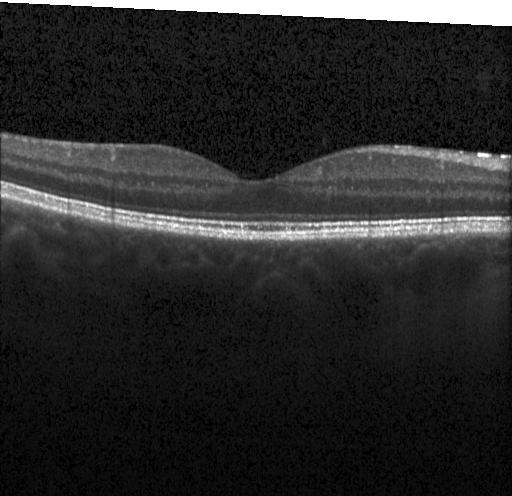

Retinal OCT B-scan; instrument: Heidelberg Spectralis — Diagnosis: no choroidal neovascularization, no diabetic macular edema, and no drusen.